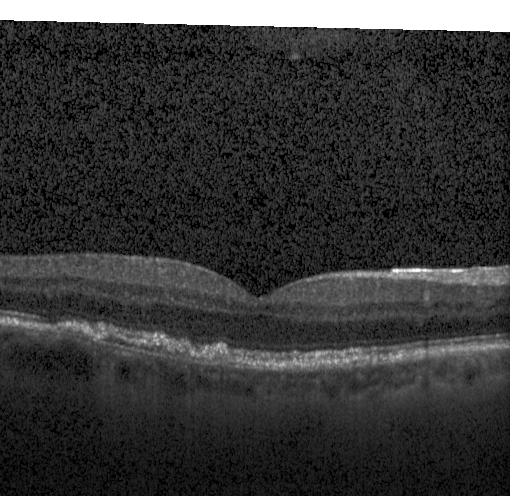 Dx: sub-RPE drusenoid deposits.